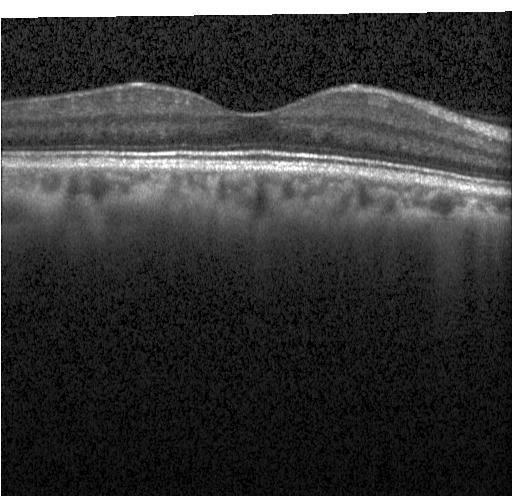
Fovea-centered · OCT line scan — Diagnosis: no choroidal neovascularization, no diabetic macular edema, and no drusen.